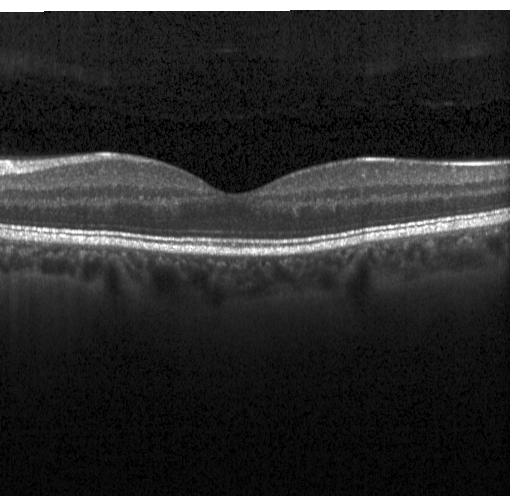

Diagnosis: no evidence of choroidal neovascularization, diabetic macular edema, or drusen.